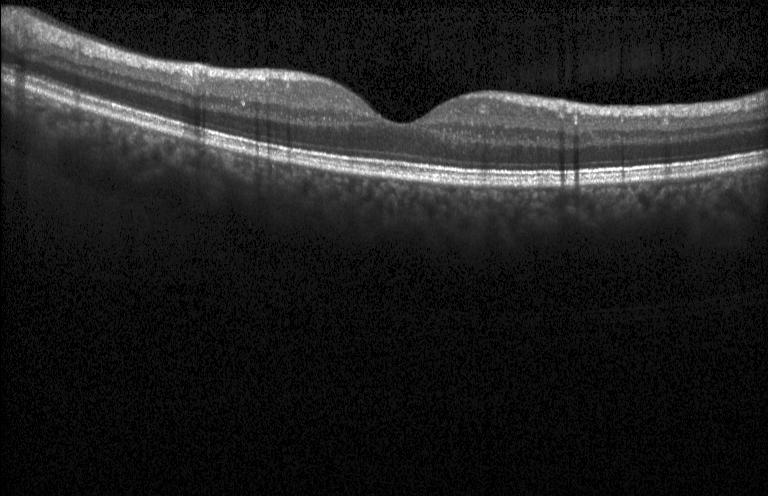

The scan shows no choroidal neovascularization, diabetic macular edema, or drusen.